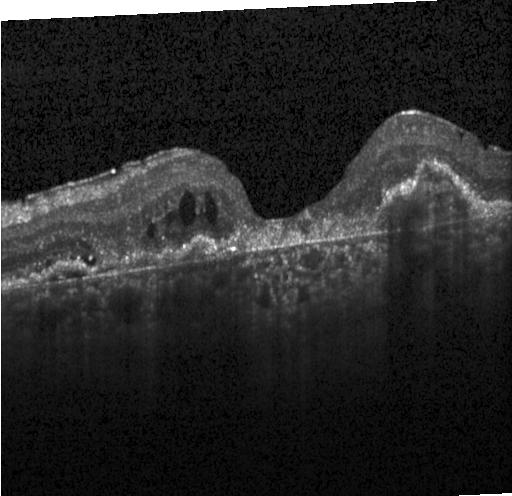

Retinal OCT cross-section
Impression: a choroidal neovascular membrane.